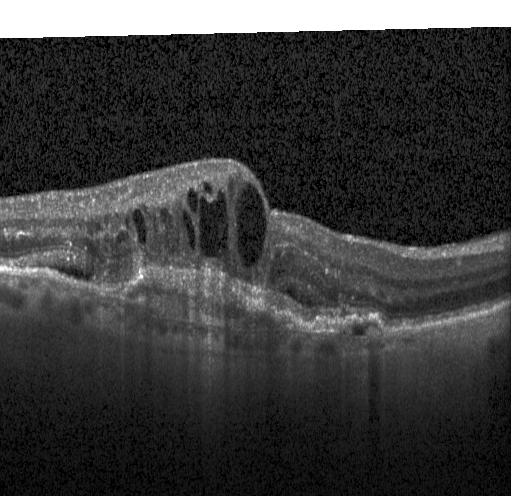

OCT finding: choroidal neovascularization (CNV).